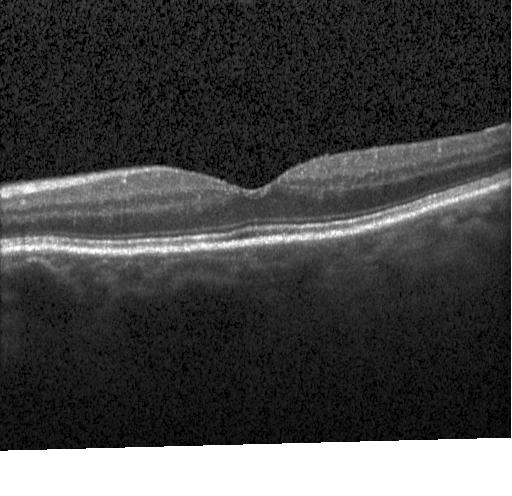 Retinal OCT B-scan, acquired on a Heidelberg Spectralis, centered on the fovea, spectral-domain OCT
The scan shows no CNV, no DME, and no drusen.